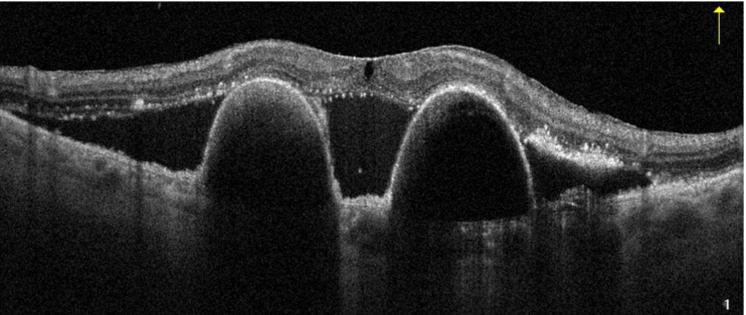

Through the macula; OCT line scan; Optovue Avanti RTVue XR — Assessment: age-related macular degeneration.